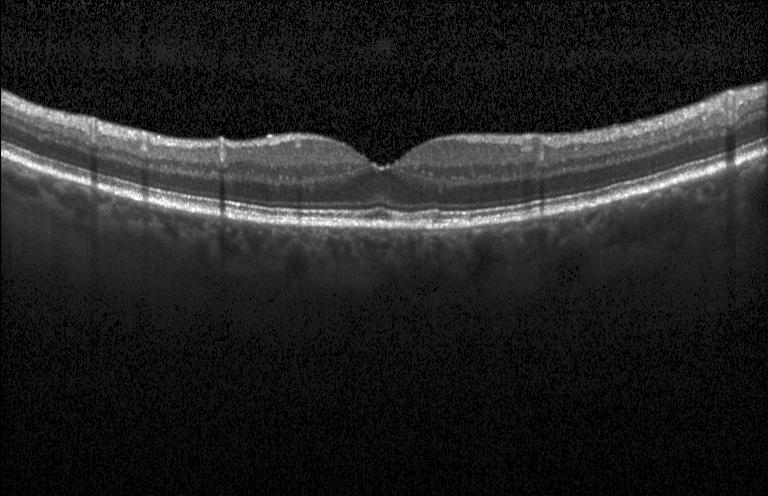 OCT B-scan · instrument: Heidelberg Spectralis · spectral-domain optical coherence tomography · horizontal scan through the fovea. Impression: neither choroidal neovascularization, diabetic macular edema, nor drusen.